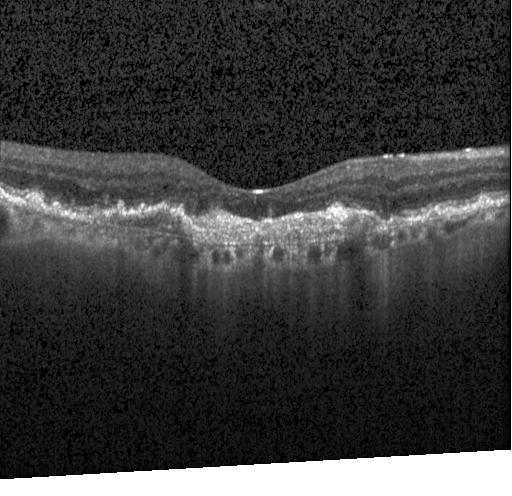 OCT B-scan showing a choroidal neovascular membrane.